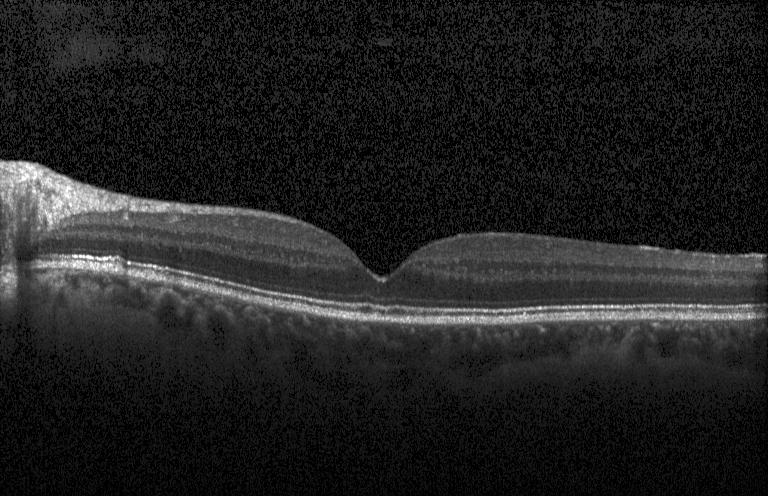
This B-scan demonstrates no evidence of CNV, DME, or drusen.